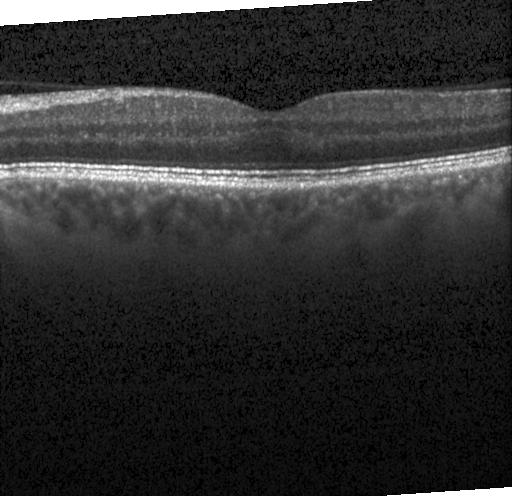 Spectral-domain optical coherence tomography; optical coherence tomography B-scan; centered on the fovea
Finding: no choroidal neovascularization, no diabetic macular edema, and no drusen.